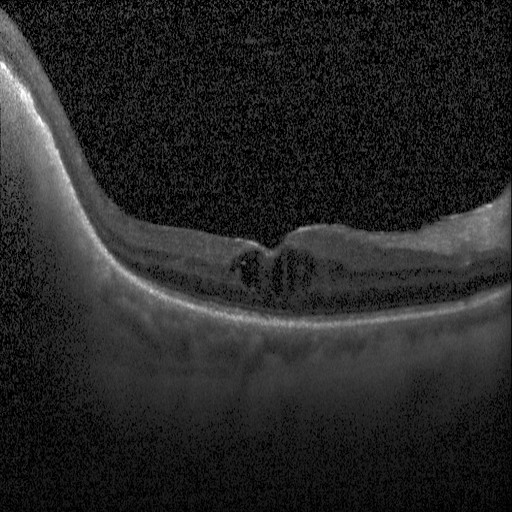 Acquired on a Heidelberg Spectralis, SD-OCT, optical coherence tomography B-scan — Impression: DME.